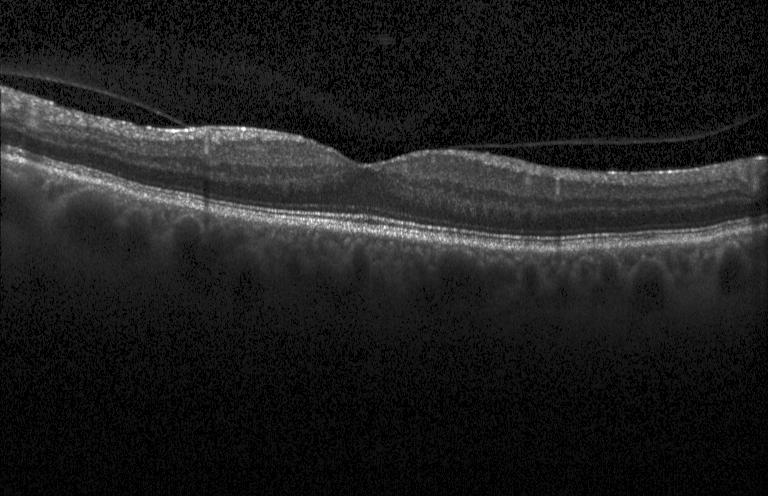 This B-scan demonstrates neither choroidal neovascularization, diabetic macular edema, nor drusen.